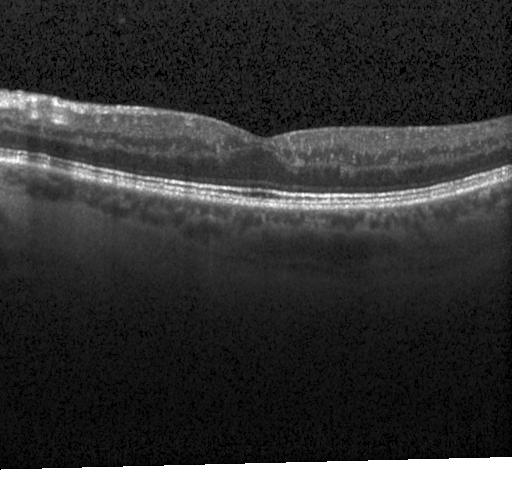 Optical coherence tomography B-scan, acquired on a Heidelberg Spectralis — Finding: no CNV, no DME, and no drusen.